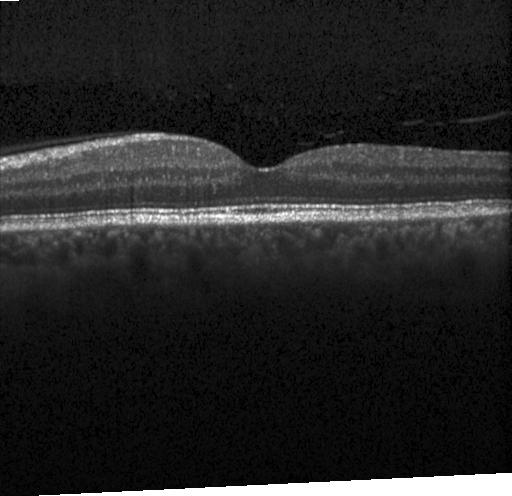
Optical coherence tomography B-scan.
Diagnosis: no choroidal neovascularization, no diabetic macular edema, and no drusen.